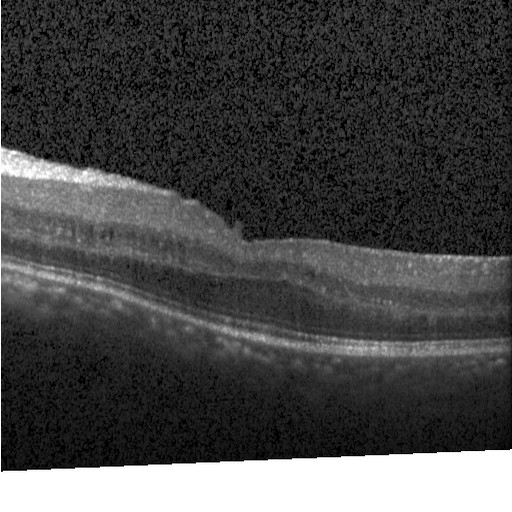
Finding: diabetic macular edema.